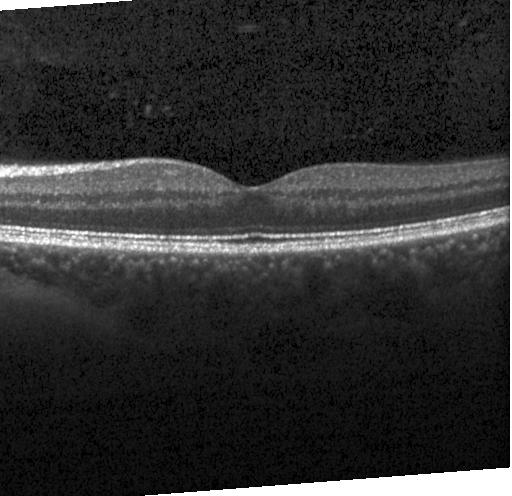
Retinal OCT B-scan, spectral-domain optical coherence tomography, centered on the fovea.
Finding: no evidence of choroidal neovascularization, diabetic macular edema, or drusen.